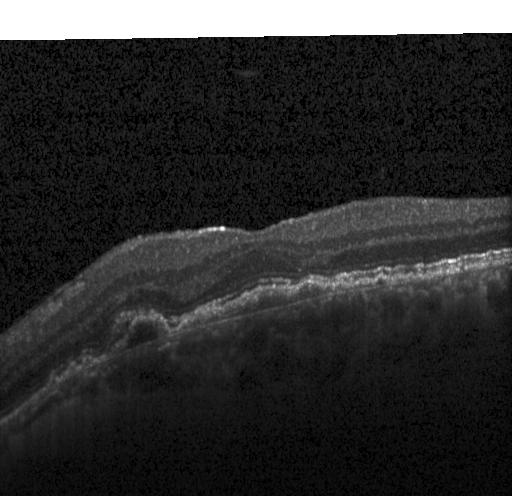
Spectral-domain optical coherence tomography, optical coherence tomography scan.
Macular OCT: CNV.